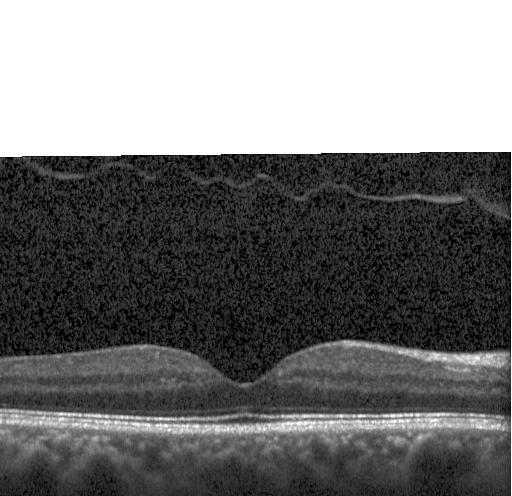
Retinal OCT cross-section. Assessment: neither choroidal neovascularization, diabetic macular edema, nor drusen.